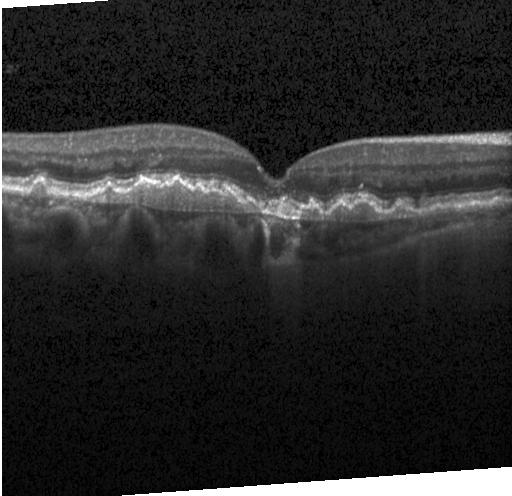 Impression: choroidal neovascularization.